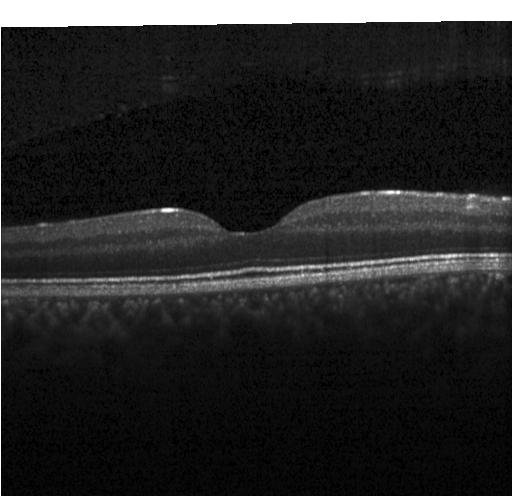 OCT B-scan. Spectral-domain OCT — This B-scan demonstrates neither choroidal neovascularization, diabetic macular edema, nor drusen.